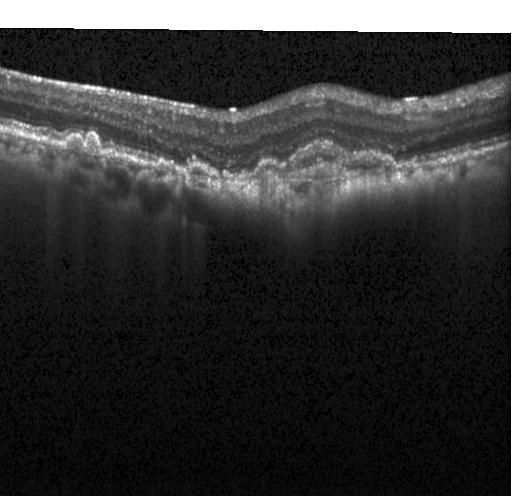

OCT finding: a choroidal neovascular membrane.